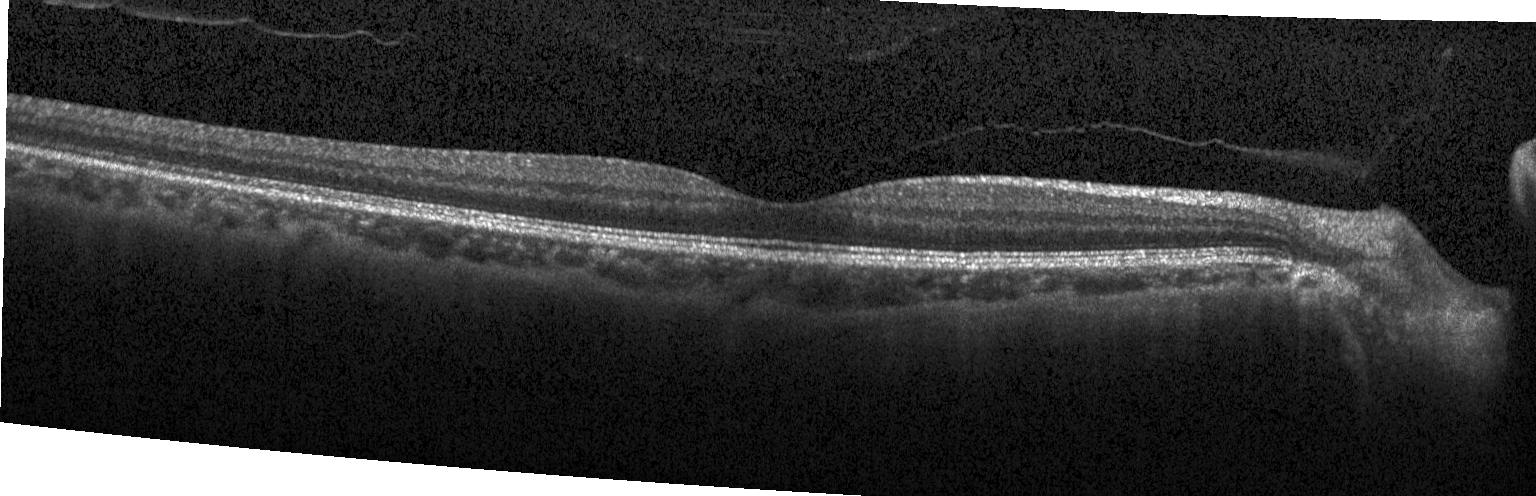 Spectral-domain OCT, retinal OCT B-scan, Heidelberg Spectralis OCT system. Assessment: no evidence of choroidal neovascularization, diabetic macular edema, or drusen.